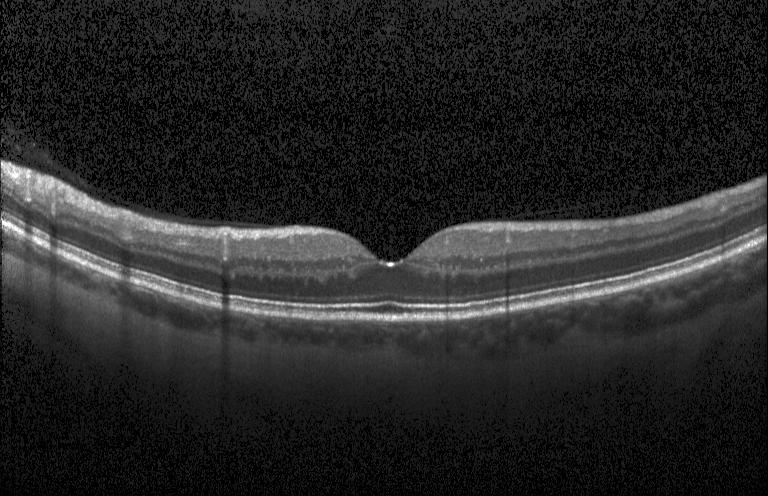 Optical coherence tomography B-scan
Macular OCT: no CNV, no DME, and no drusen.